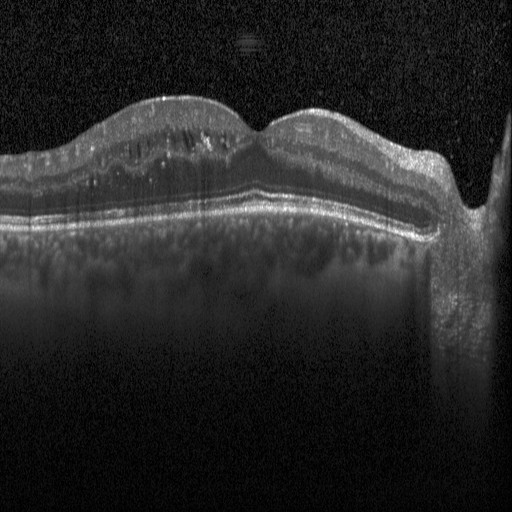 Spectral-domain optical coherence tomography · acquired on a Heidelberg Spectralis · retinal OCT cross-section. Dx: DME.